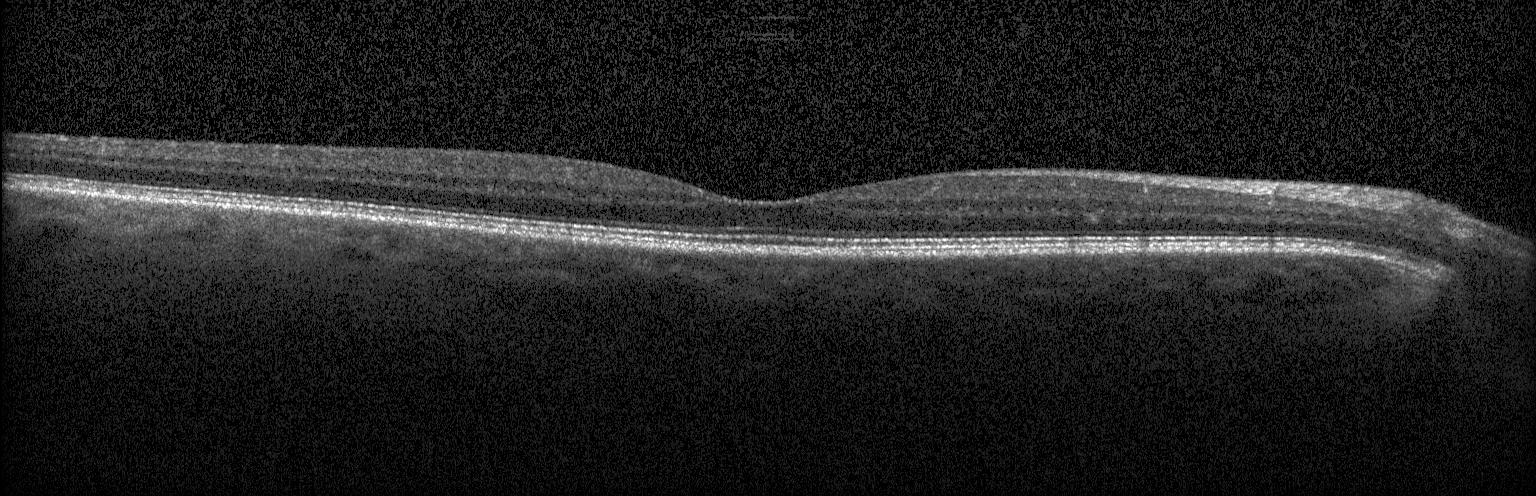

Spectral-domain OCT B-scan: no choroidal neovascularization, diabetic macular edema, or drusen.